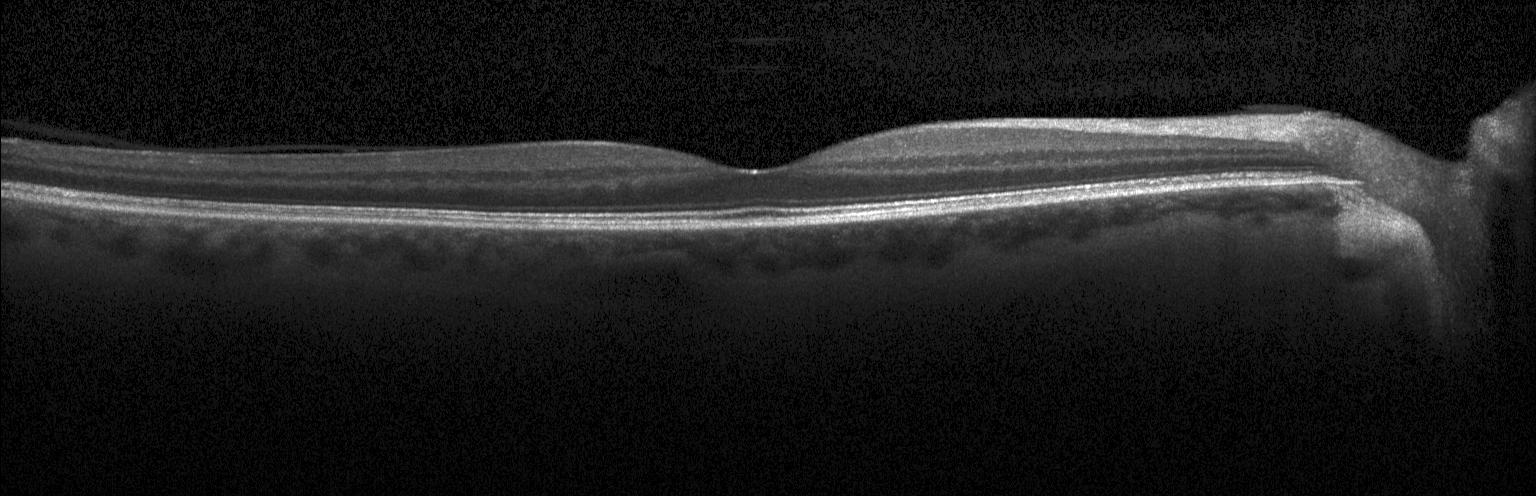 Macular OCT: no choroidal neovascularization, diabetic macular edema, or drusen.